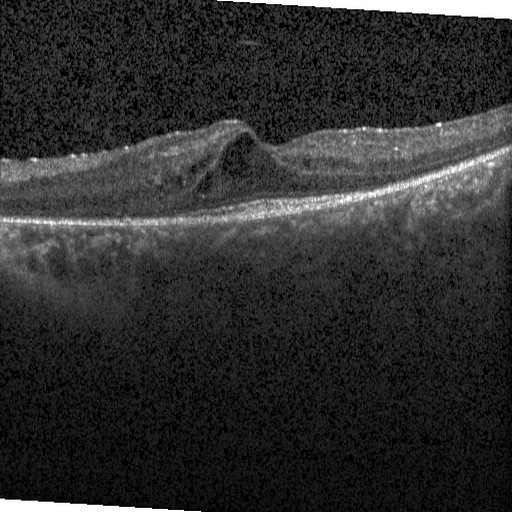 Spectral-domain OCT · optical coherence tomography B-scan · instrument: Heidelberg Spectralis.
Finding: diabetic macular edema.